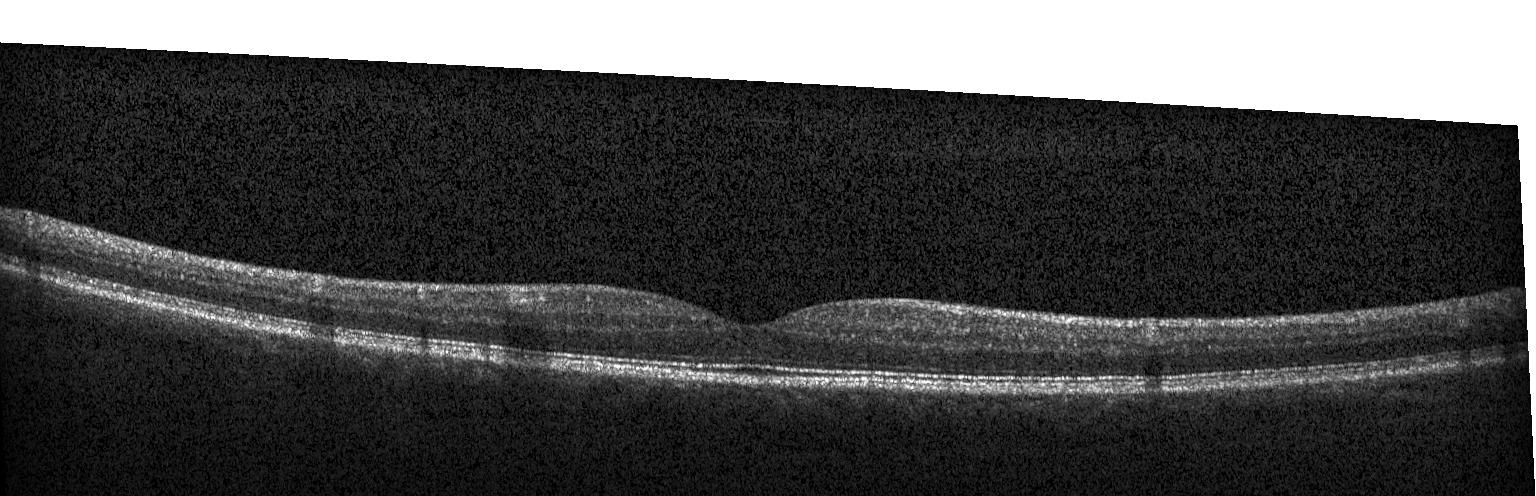

Retinal OCT B-scan. Instrument: Heidelberg Spectralis. Horizontal scan through the fovea. Assessment: neither choroidal neovascularization, diabetic macular edema, nor drusen.